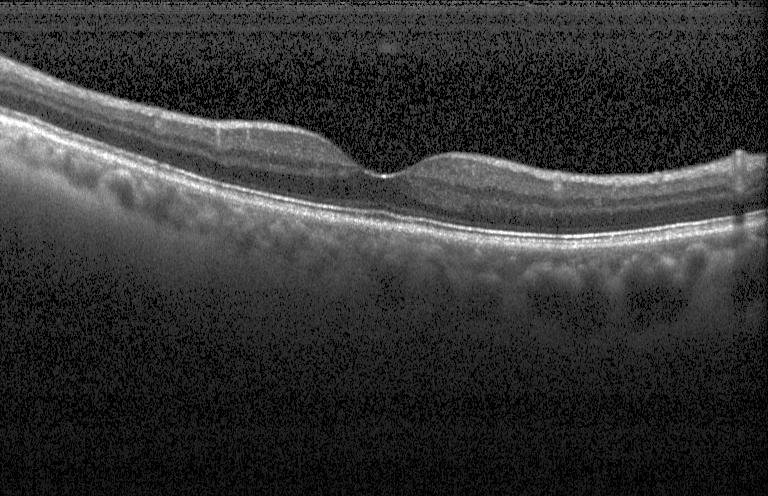

Assessment: no choroidal neovascularization, no diabetic macular edema, and no drusen.